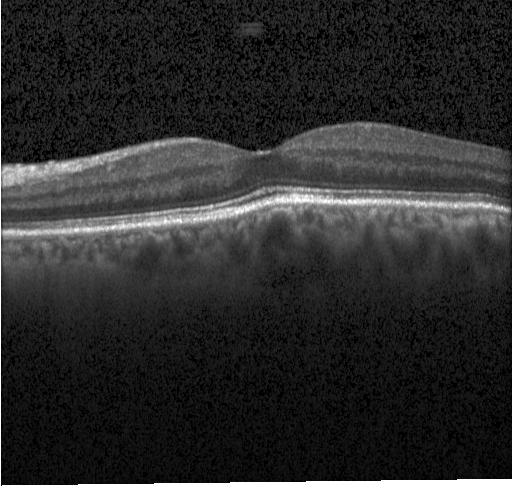 Impression: neither choroidal neovascularization, diabetic macular edema, nor drusen.